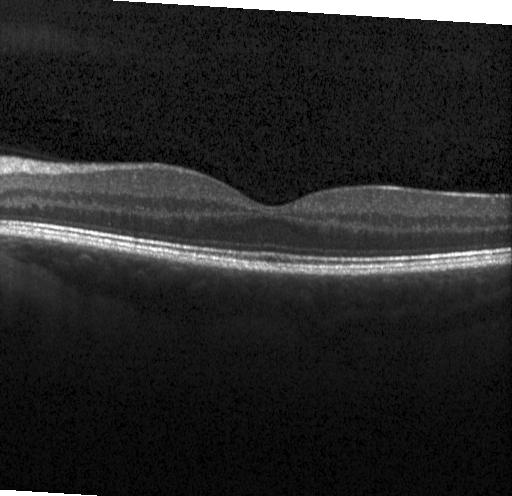
Retinal OCT B-scan · macular scan · spectral-domain optical coherence tomography. Diagnosis: no choroidal neovascularization, no diabetic macular edema, and no drusen.